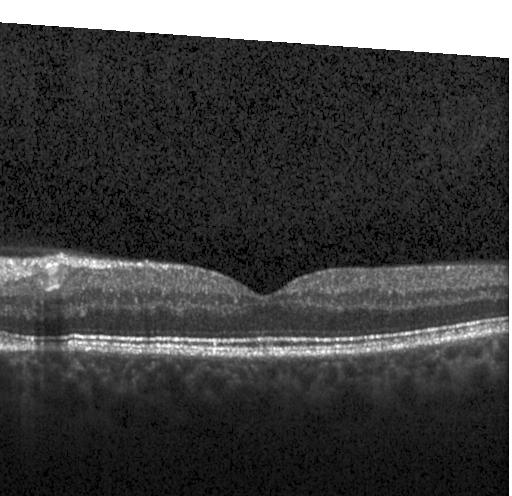 Impression: no choroidal neovascularization, no diabetic macular edema, and no drusen.